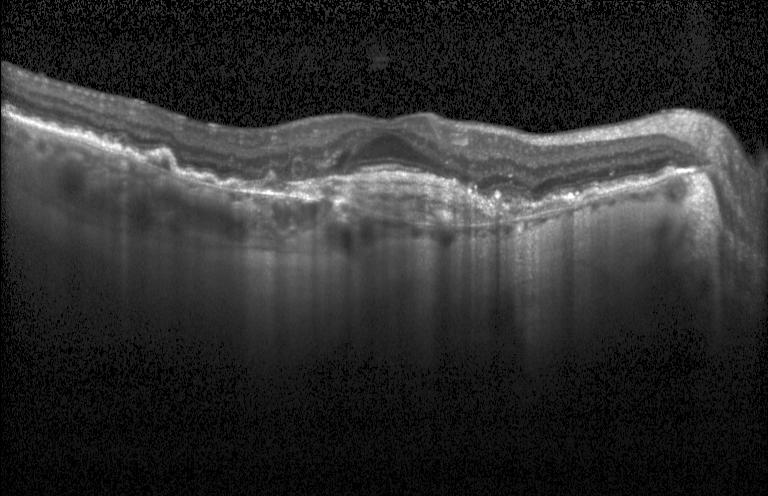

SD-OCT, macular scan, optical coherence tomography B-scan, acquired on a Heidelberg Spectralis — A choroidal neovascular membrane.